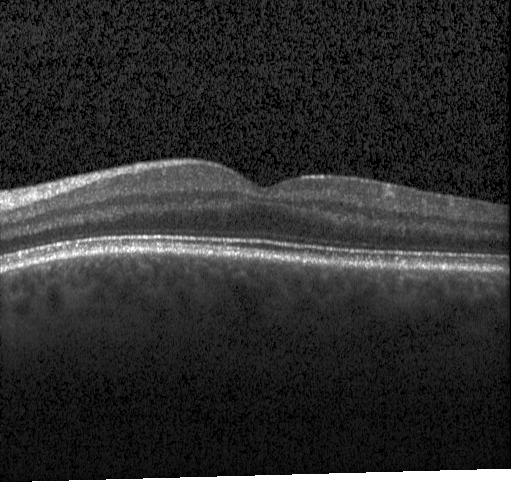

OCT B-scan.
Macular OCT: no evidence of CNV, DME, or drusen.